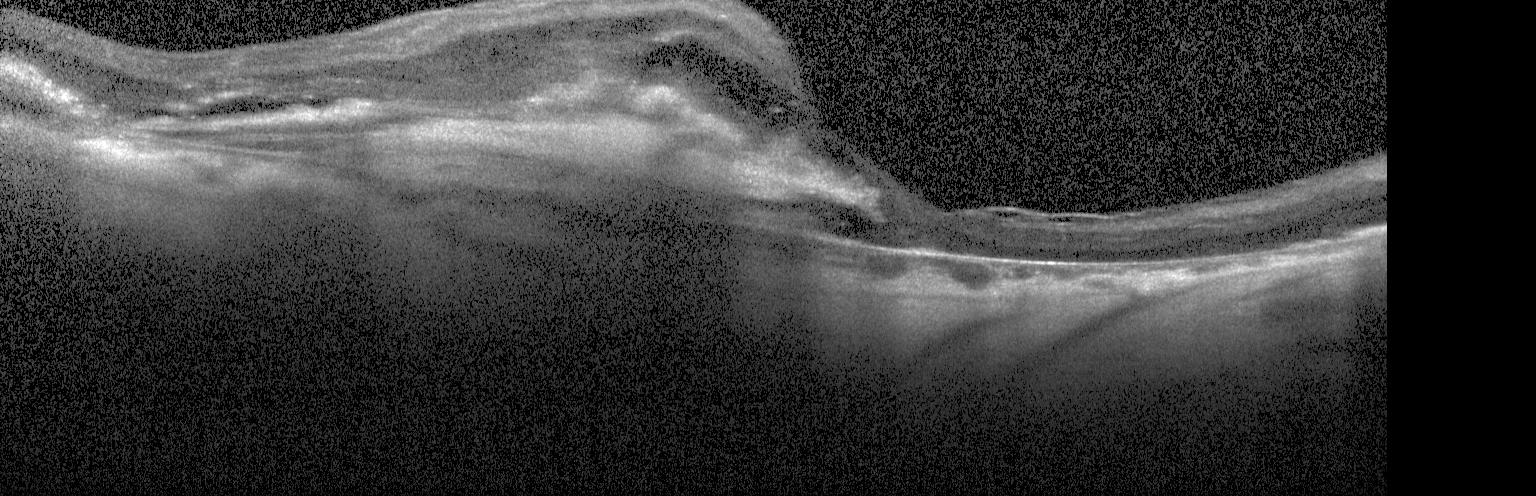 OCT line scan — Diagnosis: a choroidal neovascular membrane.